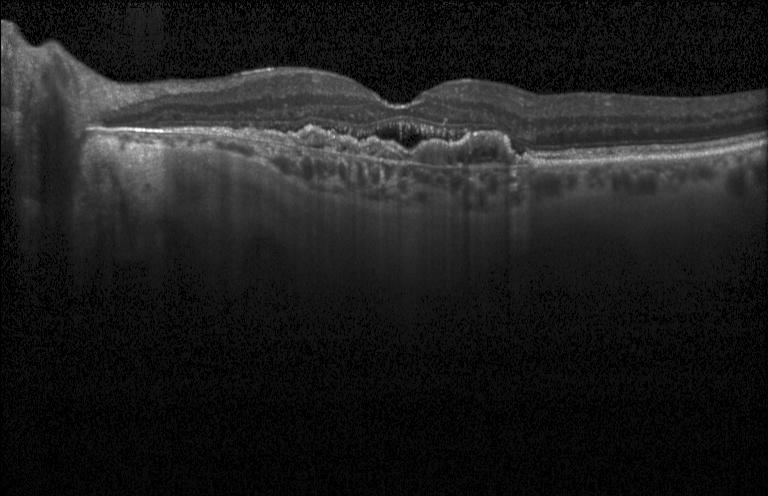
Impression: a choroidal neovascular membrane.